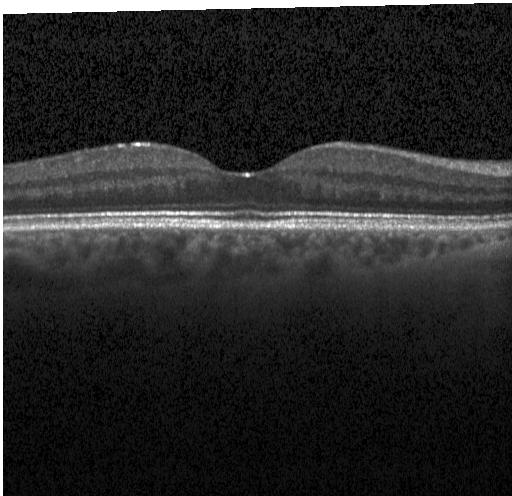

OCT B-scan, horizontal scan through the fovea, Heidelberg Spectralis OCT system, spectral-domain OCT.
Finding: neither CNV, DME, nor drusen.